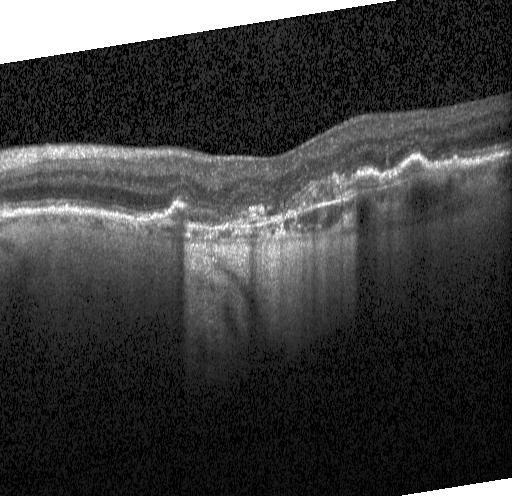

Retinal OCT B-scan
Dx: a choroidal neovascular membrane.